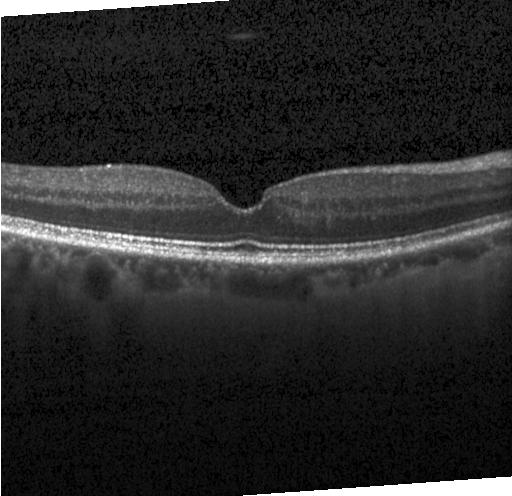 Optical coherence tomography scan · spectral-domain optical coherence tomography.
Macular OCT: no choroidal neovascularization, diabetic macular edema, or drusen.